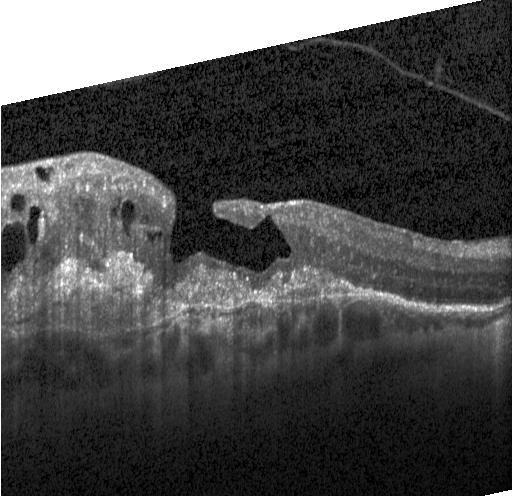
OCT B-scan; instrument: Heidelberg Spectralis; macular scan.
The scan shows choroidal neovascularization.